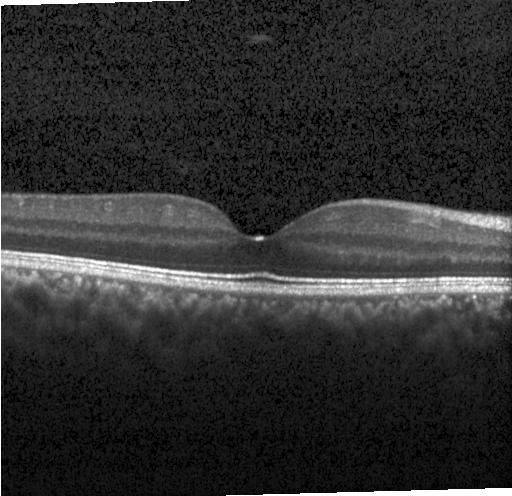
Optical coherence tomography scan, spectral-domain optical coherence tomography. Diagnosis: no CNV, no DME, and no drusen.